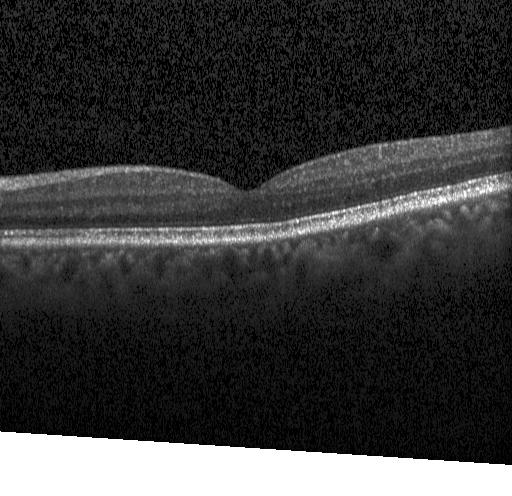 OCT finding: no evidence of choroidal neovascularization, diabetic macular edema, or drusen.